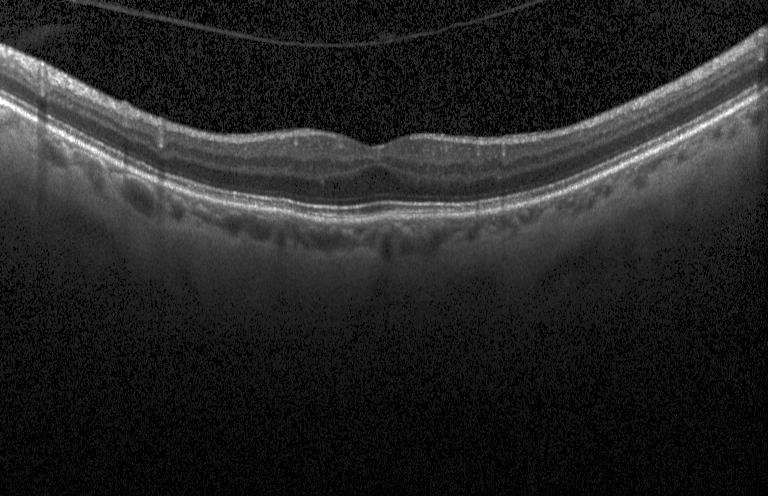

Spectral-domain OCT · optical coherence tomography scan · centered on the fovea · Heidelberg Spectralis
Finding: no CNV, no DME, and no drusen.